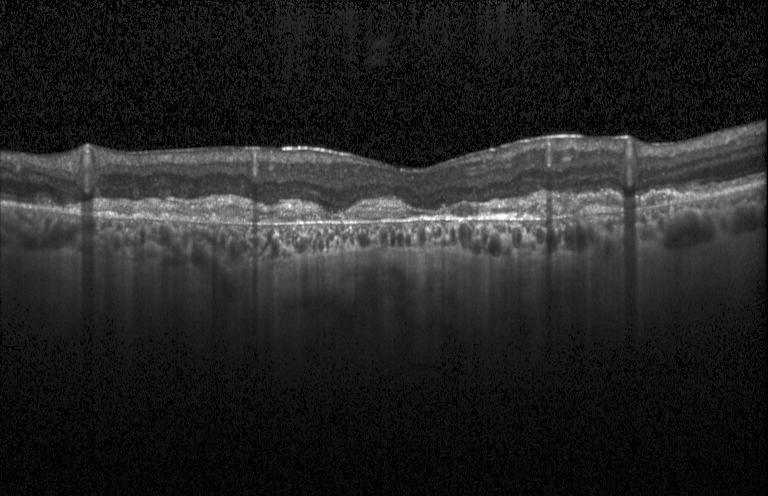 Optical coherence tomography B-scan. Impression: choroidal neovascularization.